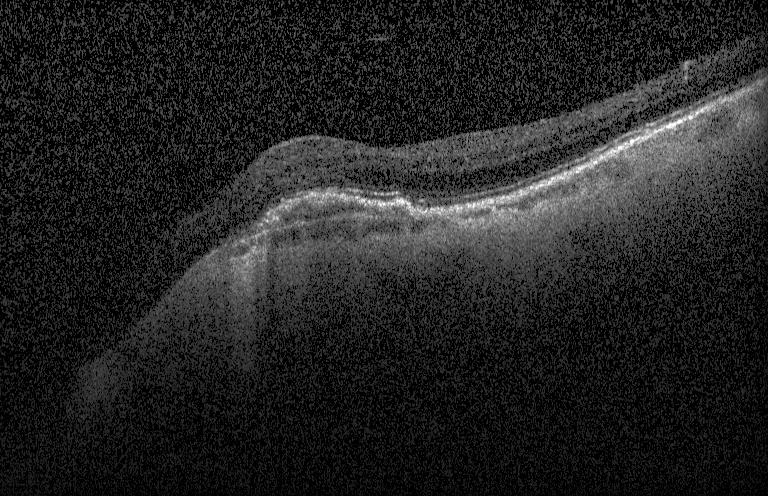
Impression: a choroidal neovascular membrane.